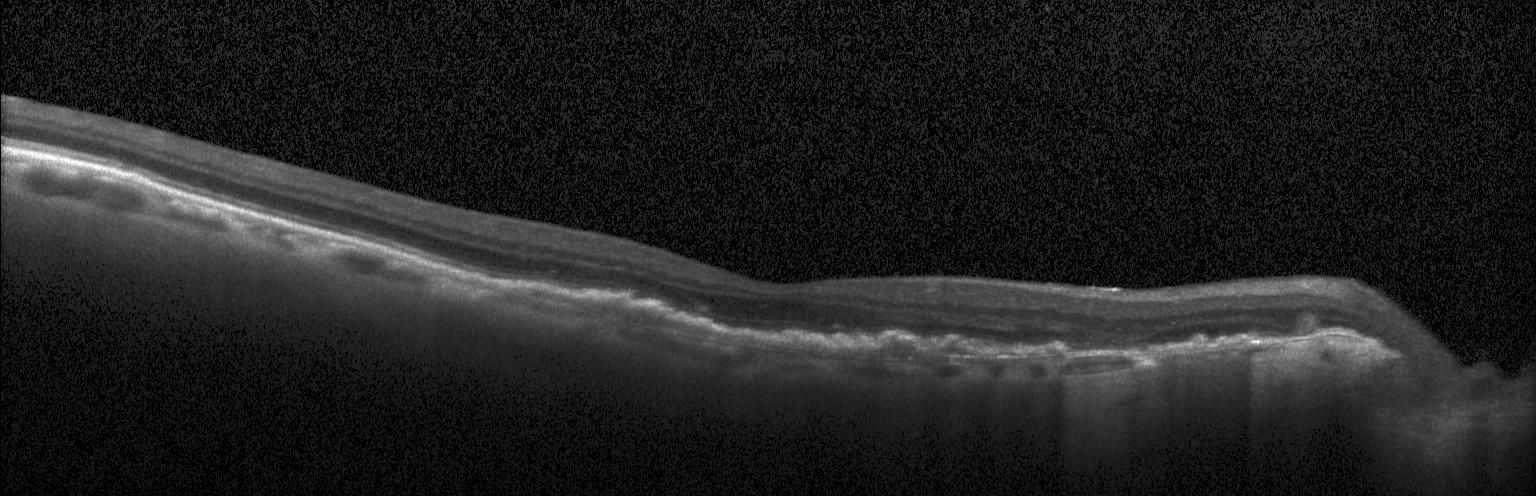
OCT scan showing choroidal neovascularization.